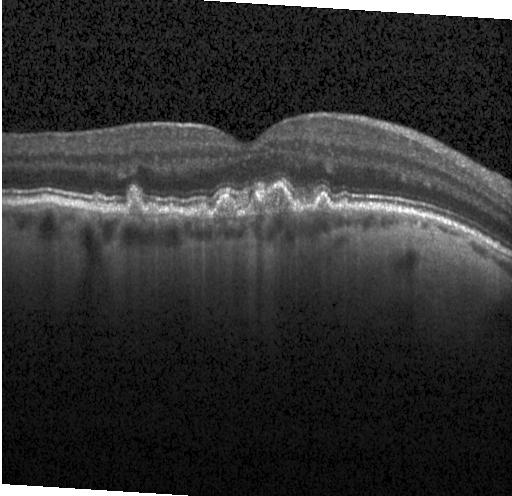

Retinal OCT cross-section showing multiple drusen.